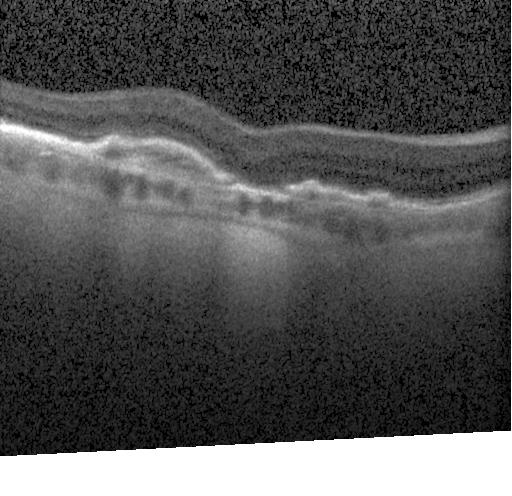
OCT finding: a choroidal neovascular membrane.